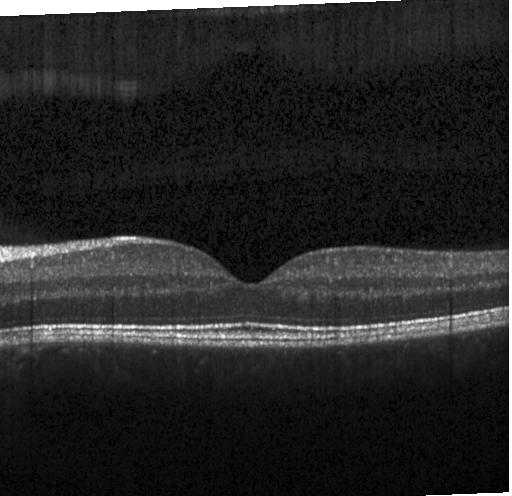

Macular OCT: no evidence of choroidal neovascularization, diabetic macular edema, or drusen.